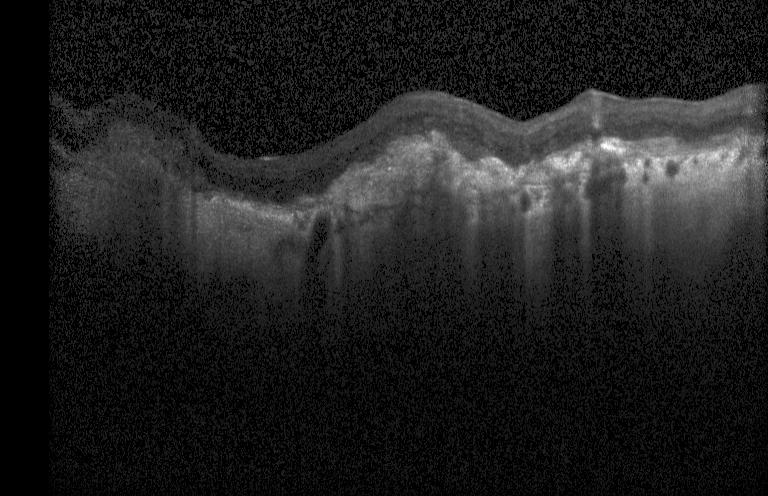
SD-OCT; optical coherence tomography B-scan; instrument: Heidelberg Spectralis; through the macula — Diagnosis: a choroidal neovascular membrane.